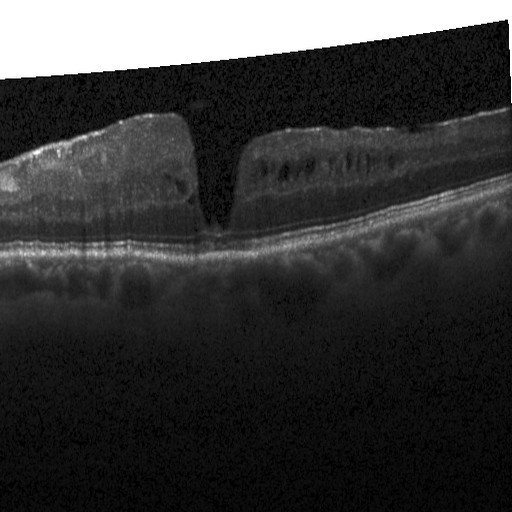 Optical coherence tomography scan. Impression: diabetic macular edema (DME).